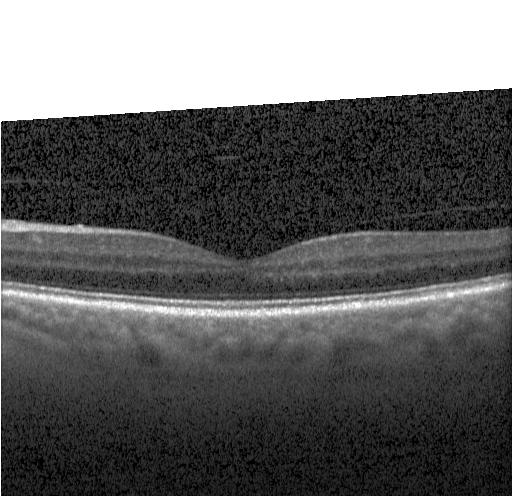
Heidelberg Spectralis OCT system, centered on the fovea, retinal OCT cross-section. Impression: no choroidal neovascularization, diabetic macular edema, or drusen.